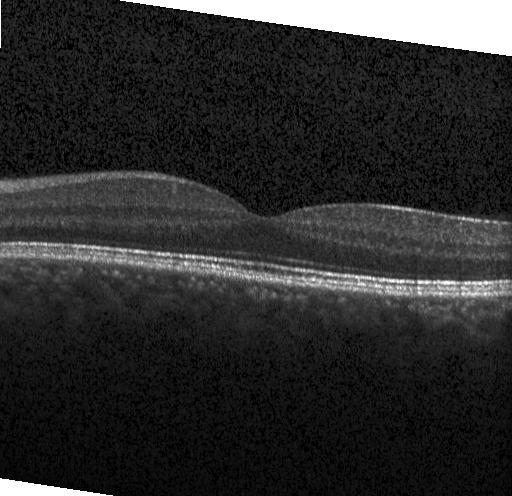 Finding: no choroidal neovascularization, no diabetic macular edema, and no drusen.